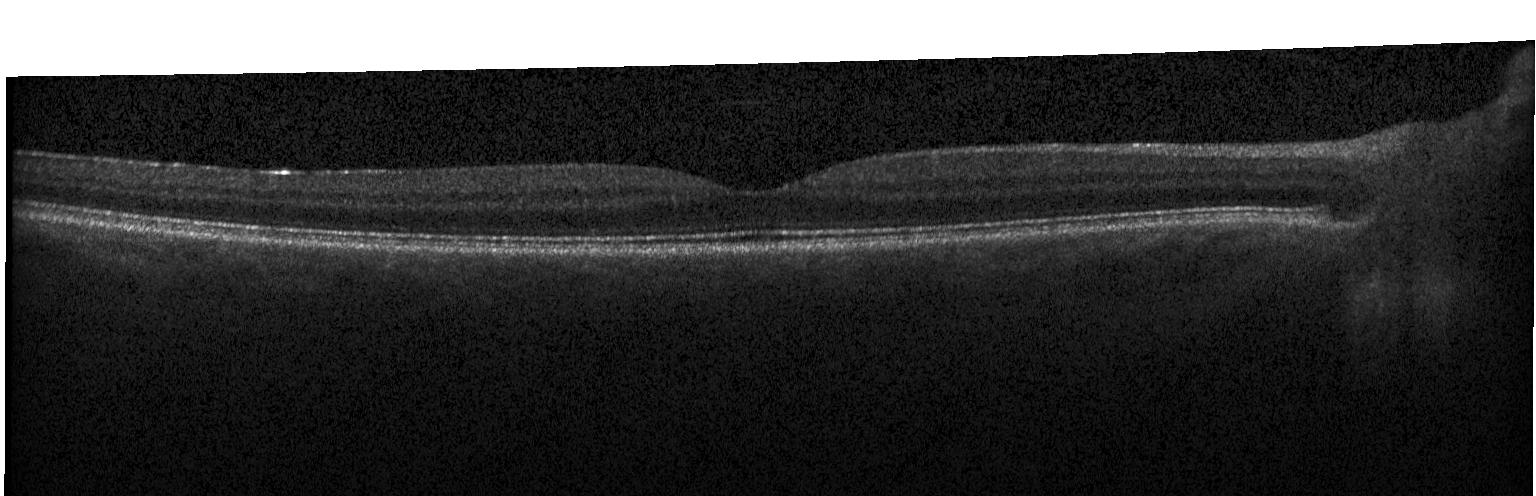

SD-OCT; OCT B-scan — No evidence of choroidal neovascularization, diabetic macular edema, or drusen.